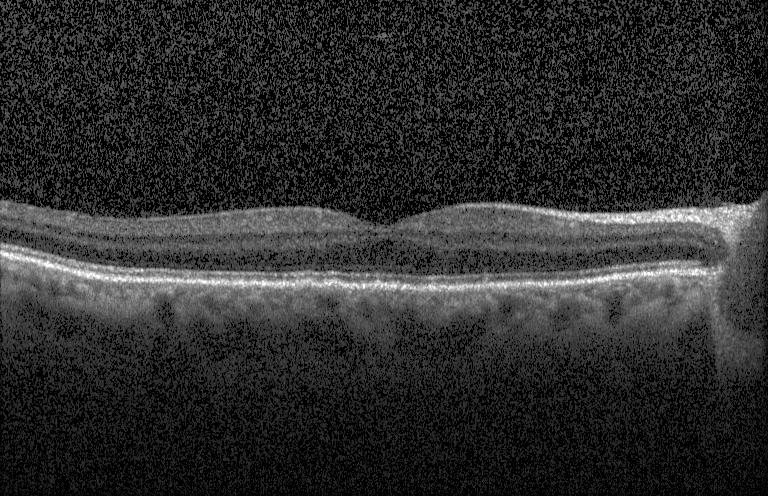

Spectral-domain optical coherence tomography. Retinal OCT cross-section. No evidence of choroidal neovascularization, diabetic macular edema, or drusen.